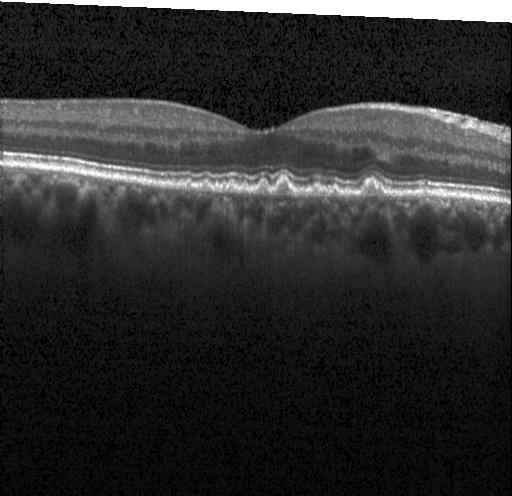 OCT line scan, Heidelberg Spectralis, through the macula, SD-OCT — Assessment: multiple drusen.